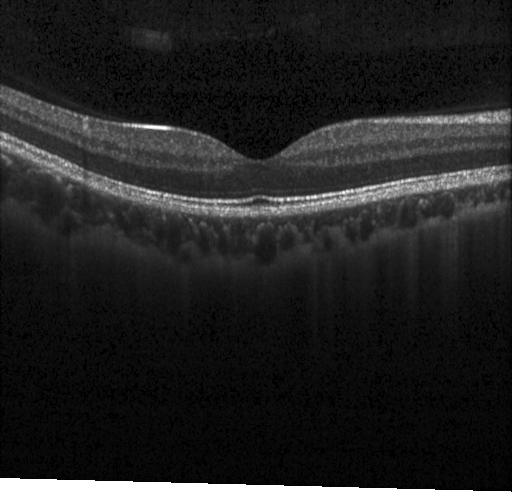
No choroidal neovascularization, diabetic macular edema, or drusen.